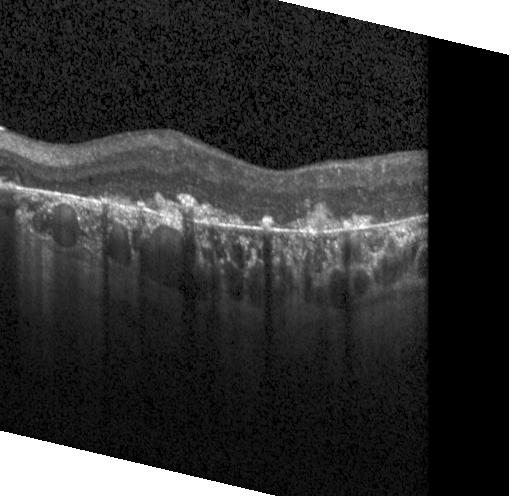

Macular OCT demonstrating a choroidal neovascular membrane.